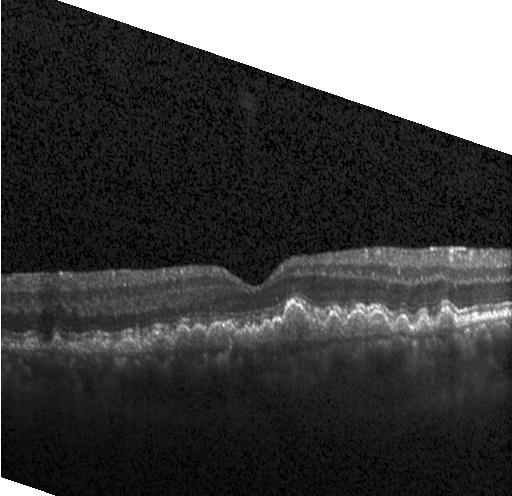 Macular OCT demonstrating a choroidal neovascular membrane.